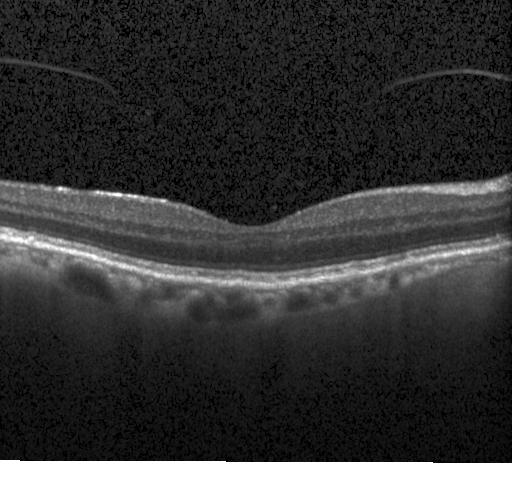
Diagnosis: neither choroidal neovascularization, diabetic macular edema, nor drusen.